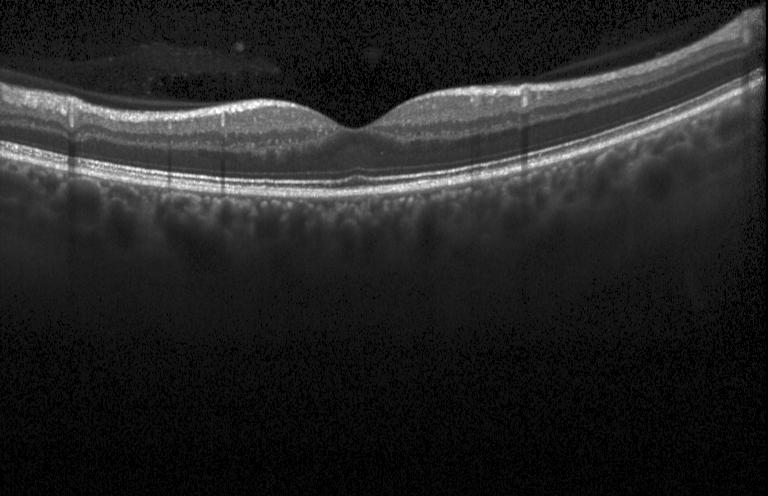 Retinal OCT cross-section.
This B-scan demonstrates no CNV, DME, or drusen.